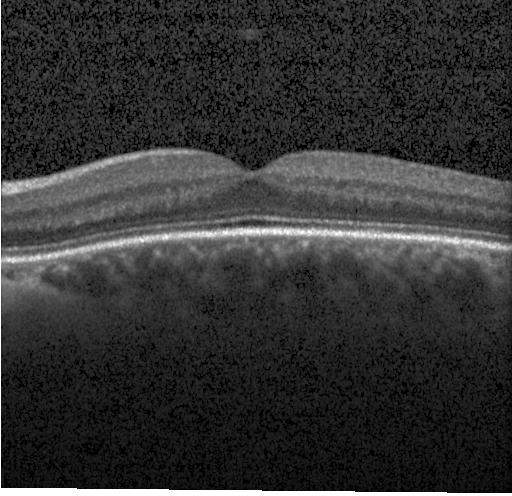 Retinal OCT cross-section showing no choroidal neovascularization, diabetic macular edema, or drusen.